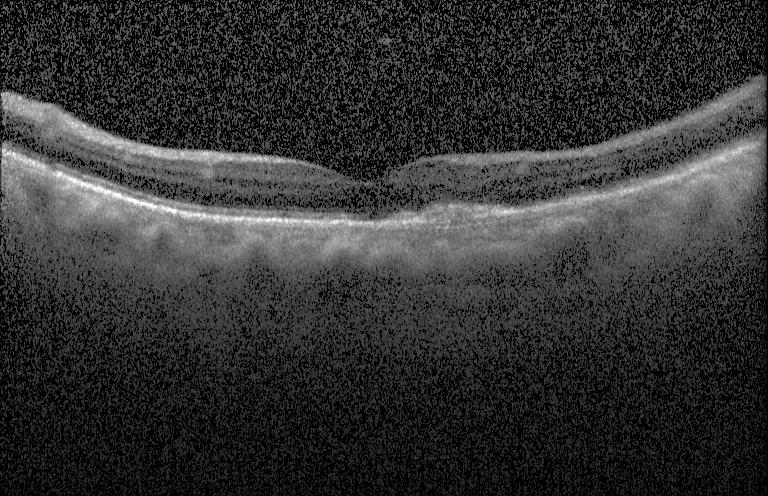 Retinal OCT cross-section showing a choroidal neovascular membrane.